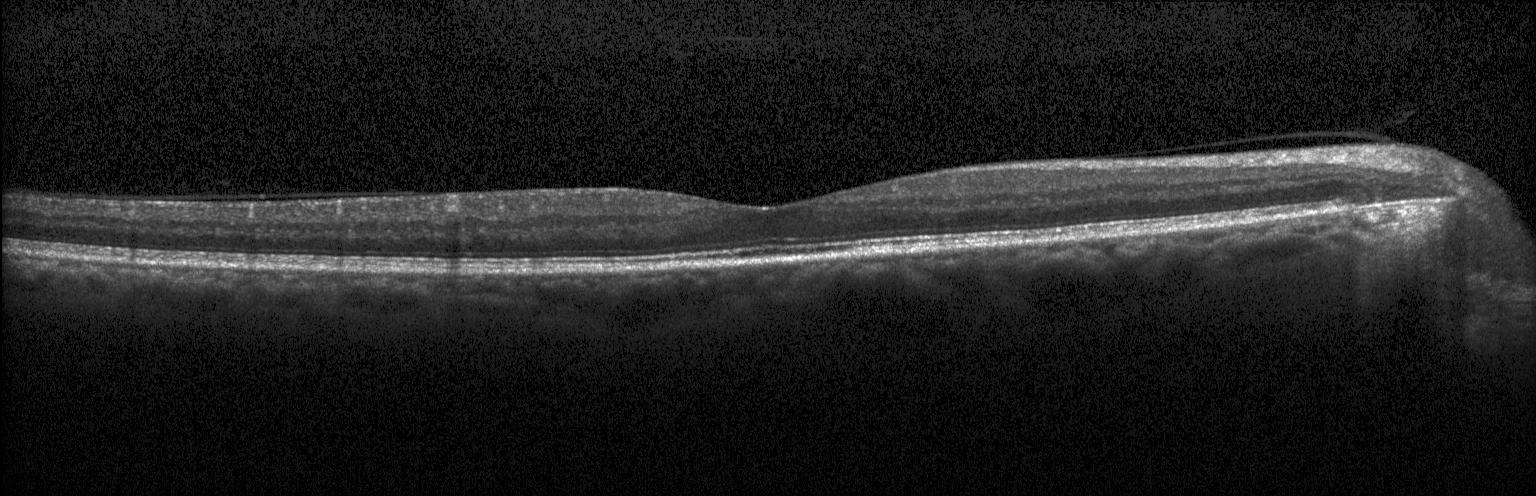 Optical coherence tomography B-scan · fovea-centered · Heidelberg Spectralis — Dx: neither choroidal neovascularization, diabetic macular edema, nor drusen.